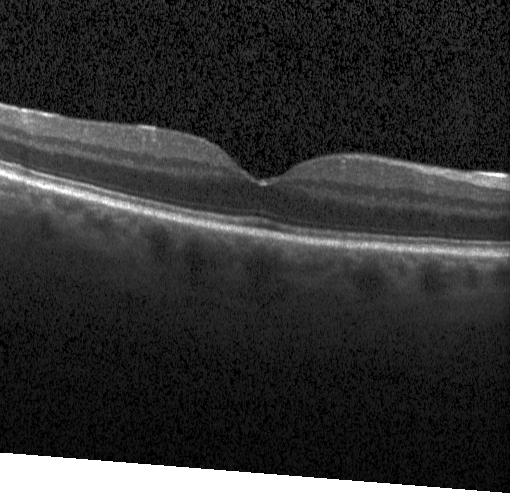

Optical coherence tomography B-scan.
This B-scan demonstrates no choroidal neovascularization, no diabetic macular edema, and no drusen.